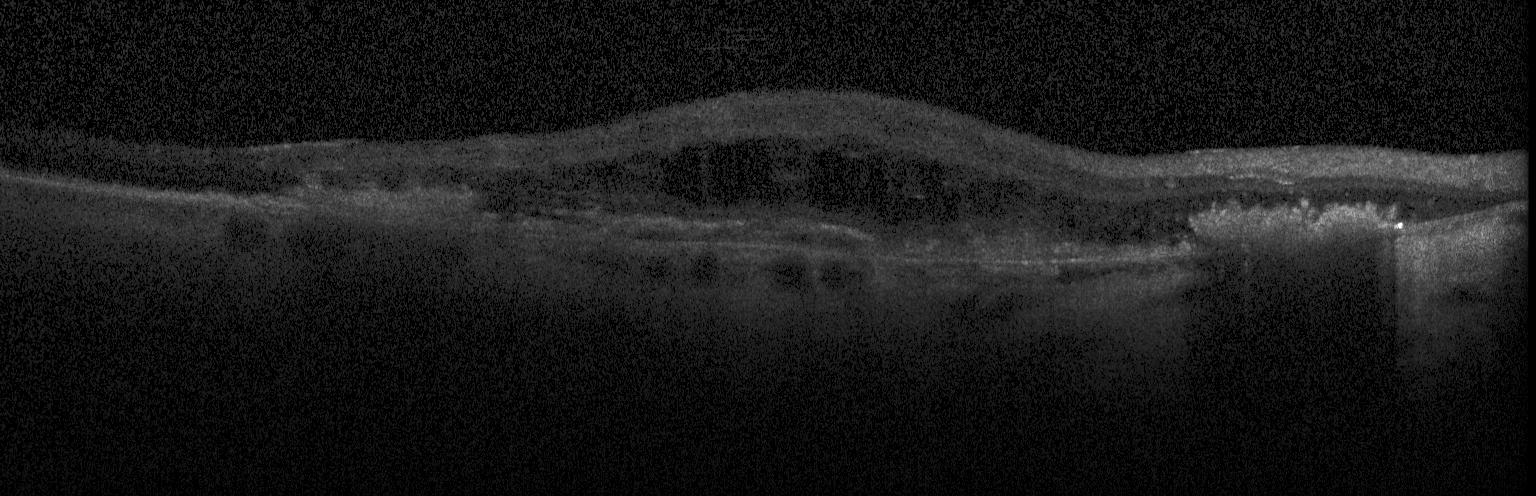 Assessment: choroidal neovascularization (CNV).